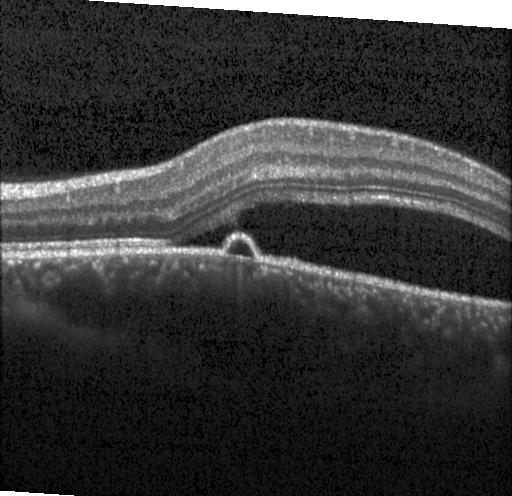 The scan shows CNV.